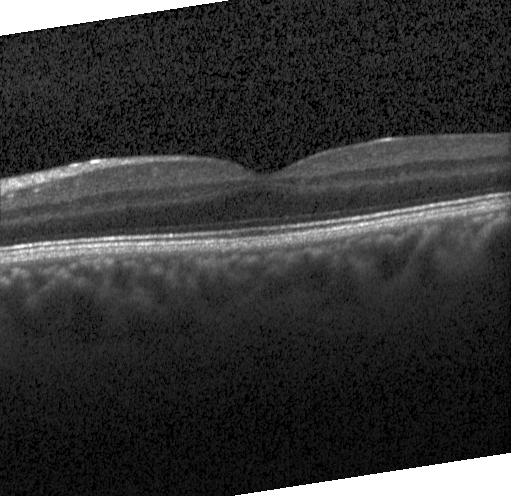

OCT B-scan.
Dx: no evidence of choroidal neovascularization, diabetic macular edema, or drusen.